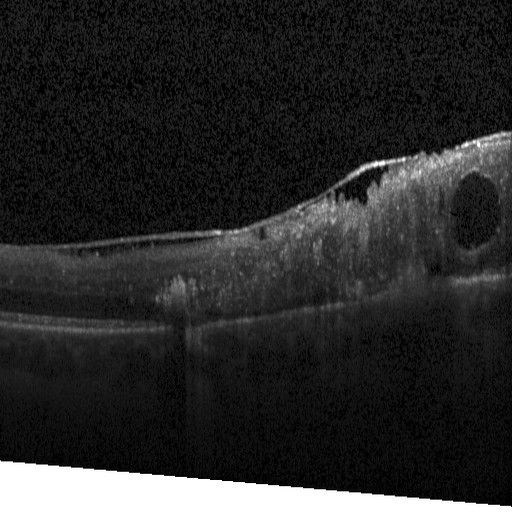
Impression: diabetic macular edema.